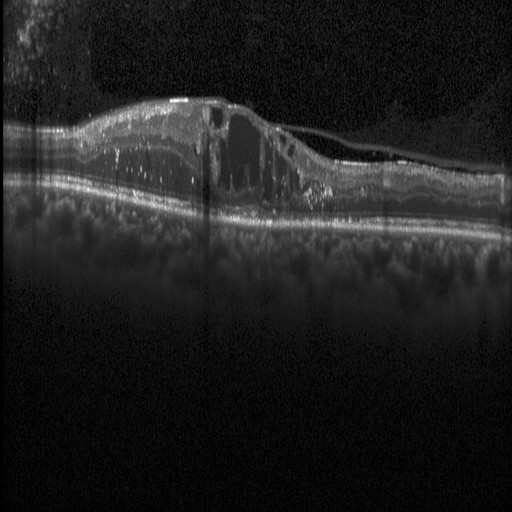

Spectral-domain OCT; OCT B-scan; instrument: Heidelberg Spectralis
Diagnosis: diabetic macular edema (DME).